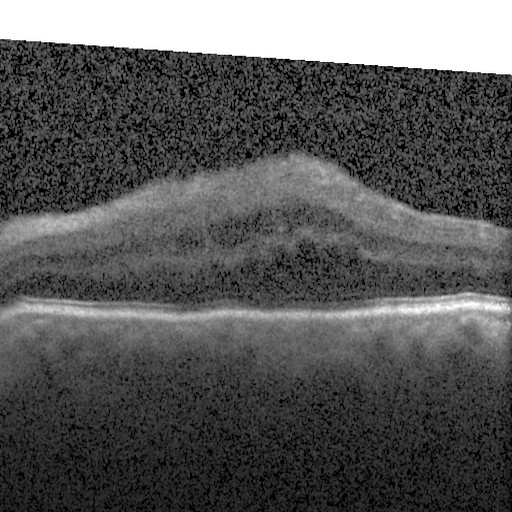

This B-scan demonstrates diabetic macular edema (DME).